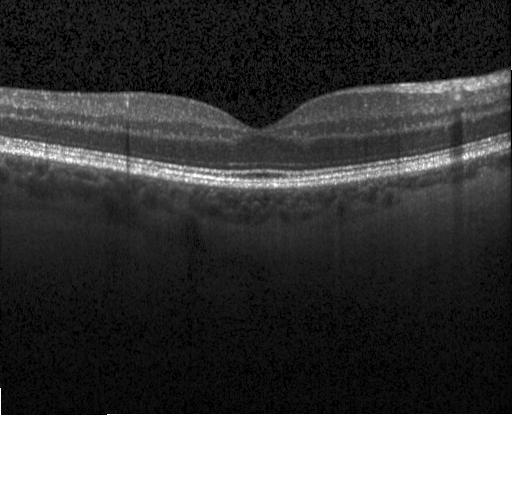 OCT line scan. Dx: no choroidal neovascularization, no diabetic macular edema, and no drusen.